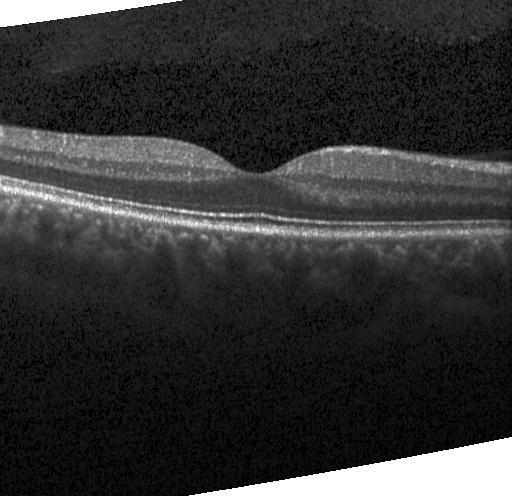

This B-scan demonstrates no choroidal neovascularization, diabetic macular edema, or drusen.